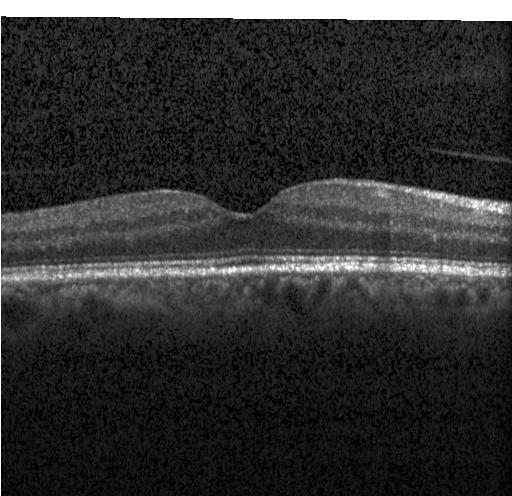

OCT finding: neither choroidal neovascularization, diabetic macular edema, nor drusen.